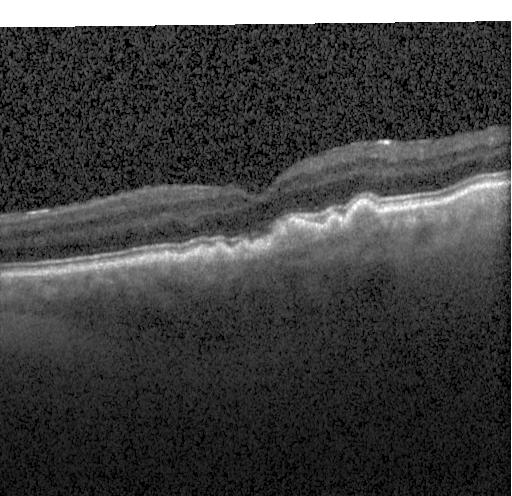
OCT scan showing multiple drusen.